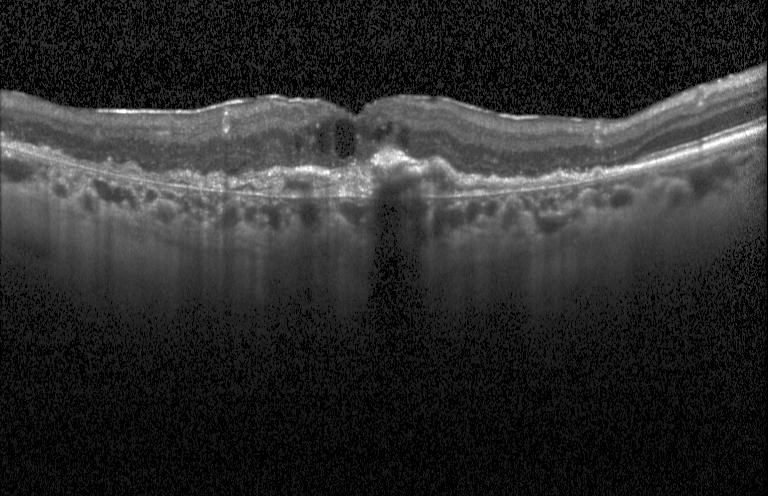

Retinal OCT B-scan · horizontal scan through the fovea. Impression: CNV.